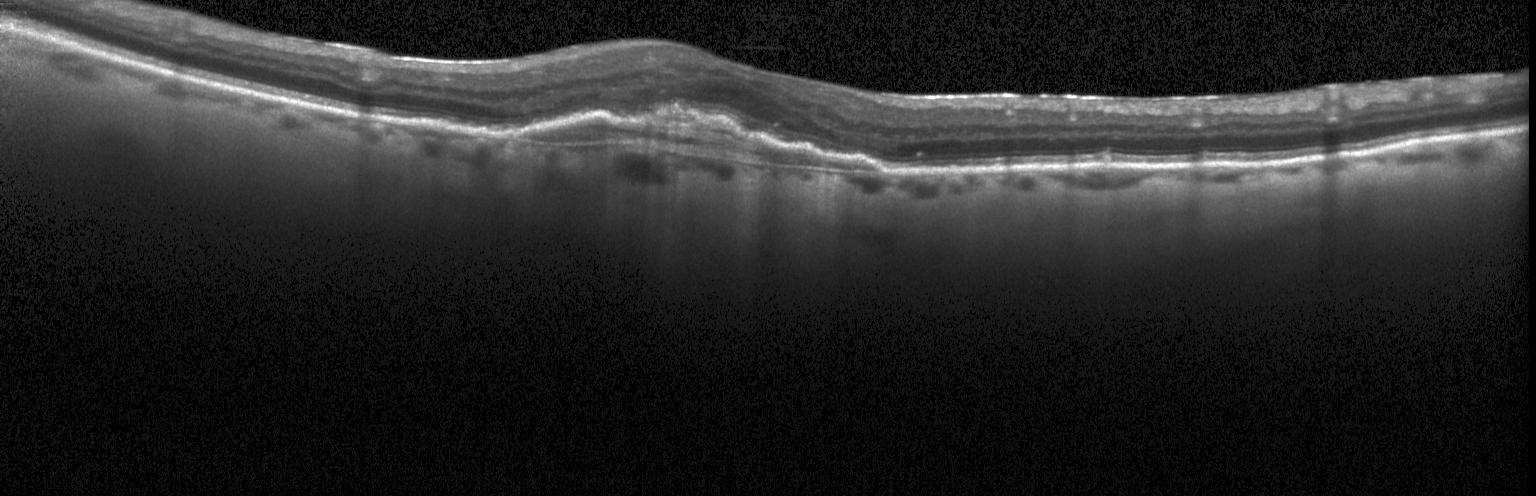

Spectral-domain optical coherence tomography, OCT line scan — Dx: choroidal neovascularization.